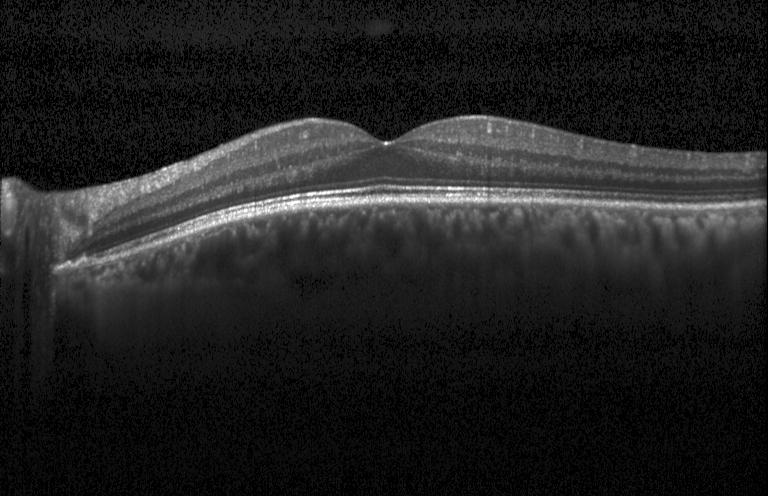
Retinal OCT cross-section; Heidelberg Spectralis; through the macula; spectral-domain OCT.
This B-scan demonstrates neither CNV, DME, nor drusen.